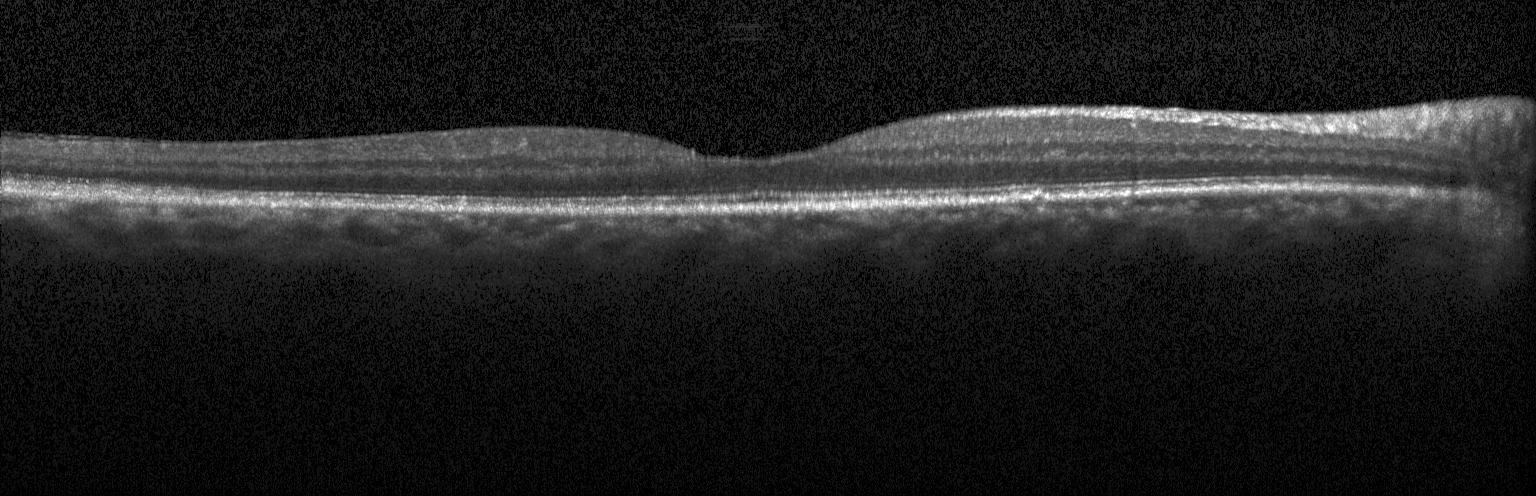

SD-OCT, optical coherence tomography B-scan, macular scan, acquired on a Heidelberg Spectralis.
The scan shows no evidence of choroidal neovascularization, diabetic macular edema, or drusen.